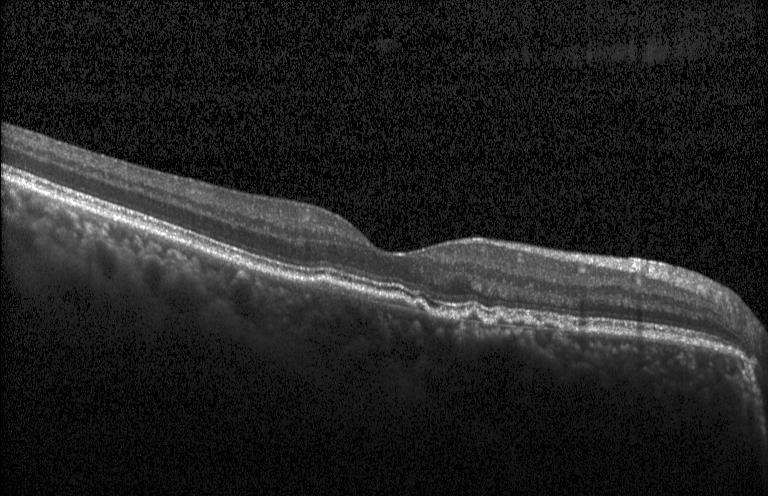

Macular scan · retinal OCT B-scan · Heidelberg Spectralis OCT system · spectral-domain OCT — This B-scan demonstrates drusen.